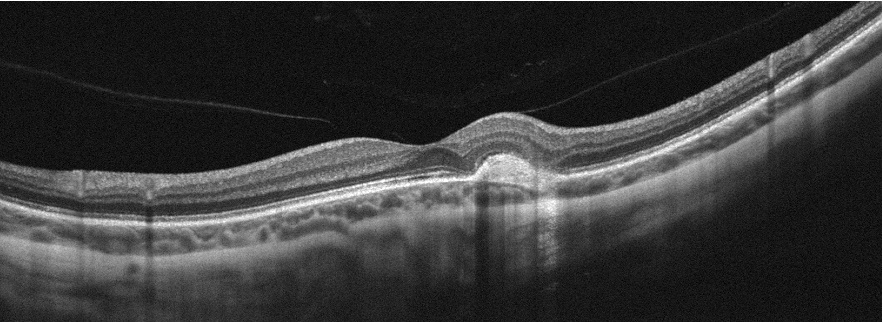 Fovea-centered. OCT line scan. Finding: age-related macular degeneration.